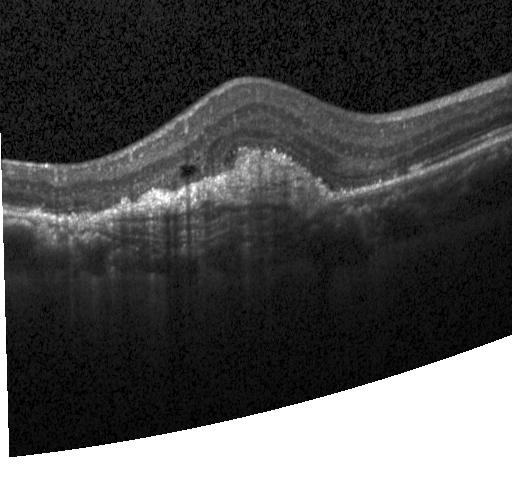

Finding: a choroidal neovascular membrane.